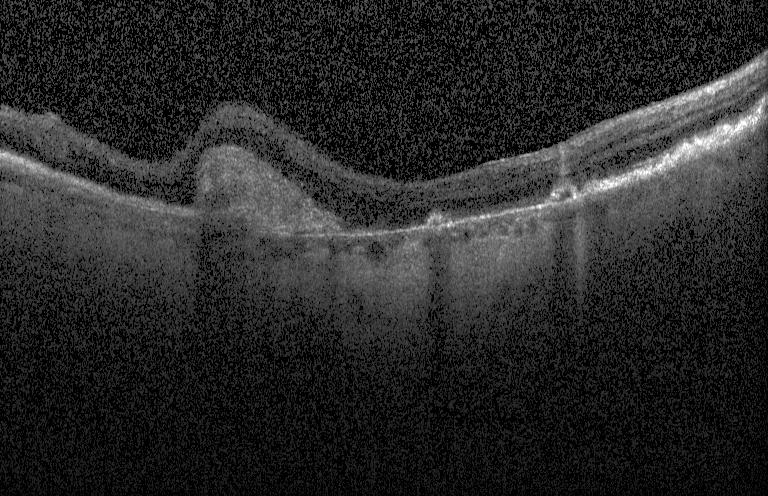
Retinal OCT cross-section; Heidelberg Spectralis; horizontal scan through the fovea; spectral-domain OCT. Diagnosis: a choroidal neovascular membrane.